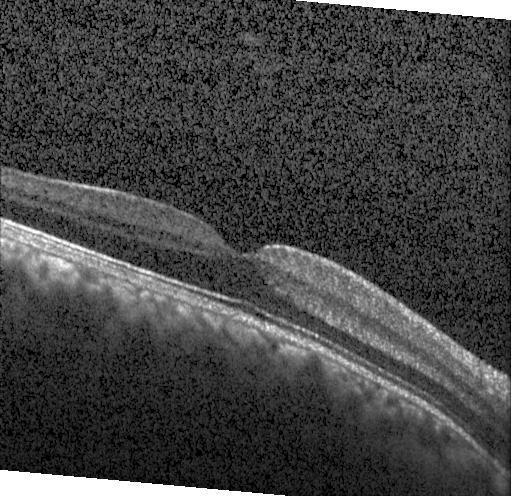
Impression: no choroidal neovascularization, no diabetic macular edema, and no drusen.